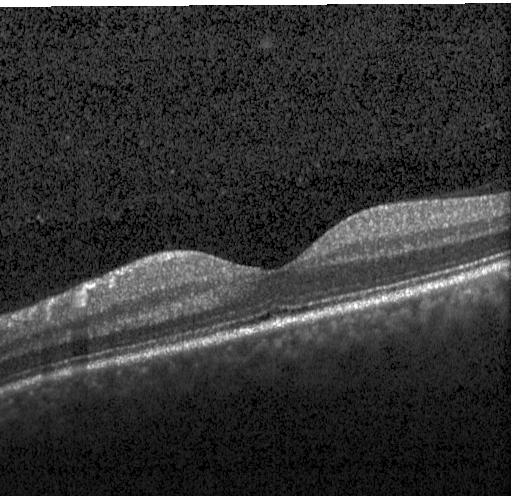 Neither CNV, DME, nor drusen.